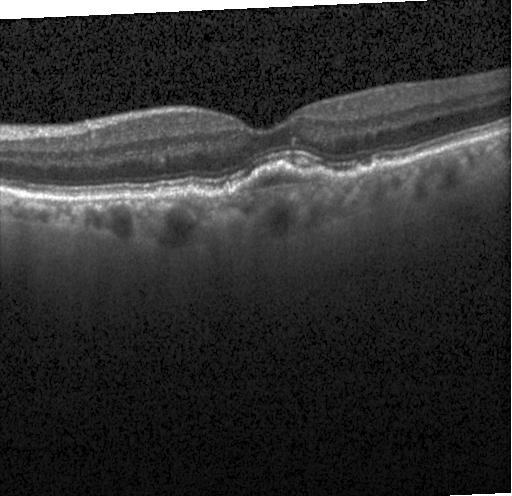

OCT B-scan showing a choroidal neovascular membrane.